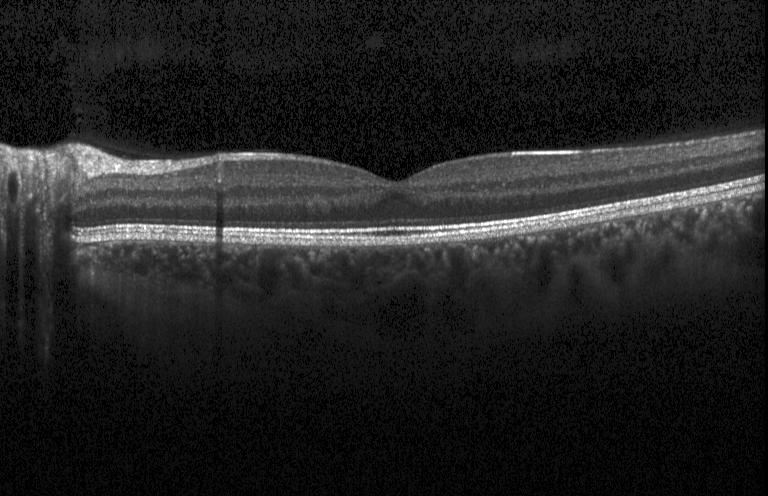
OCT B-scan, instrument: Heidelberg Spectralis, through the macula, spectral-domain optical coherence tomography — Assessment: no evidence of choroidal neovascularization, diabetic macular edema, or drusen.